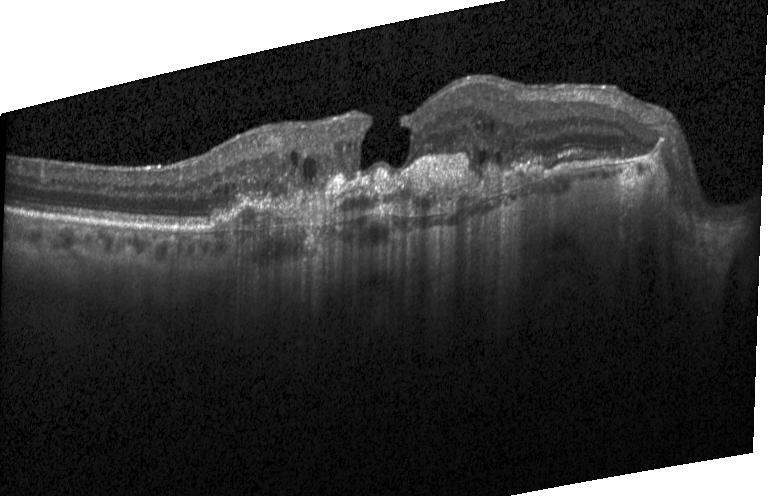 Finding: a choroidal neovascular membrane.